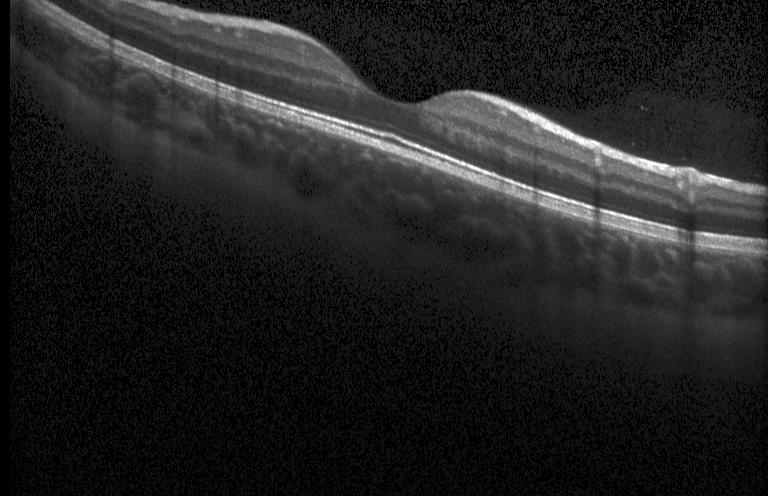
Heidelberg Spectralis; spectral-domain optical coherence tomography; fovea-centered; retinal OCT B-scan
Finding: no CNV, DME, or drusen.